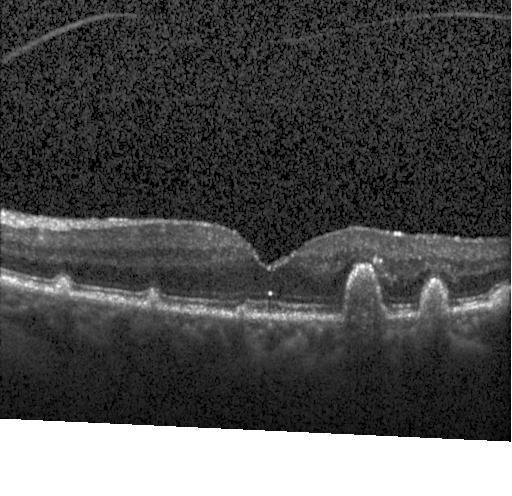

Impression: sub-RPE drusenoid deposits.